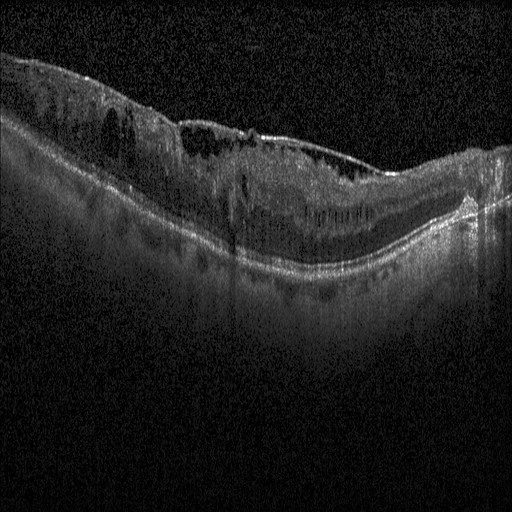

Instrument: Heidelberg Spectralis; retinal OCT B-scan; centered on the fovea. Finding: diabetic macular edema (DME).